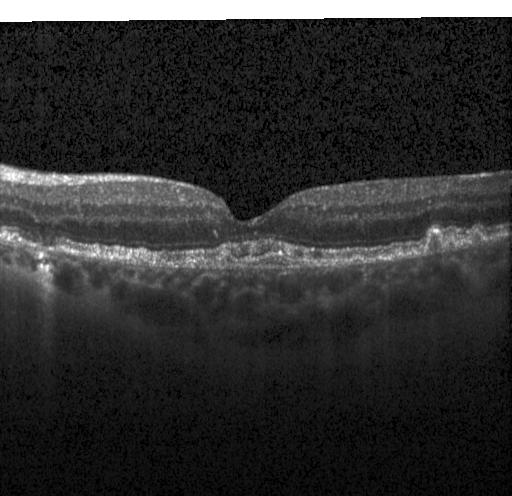

Impression: CNV.